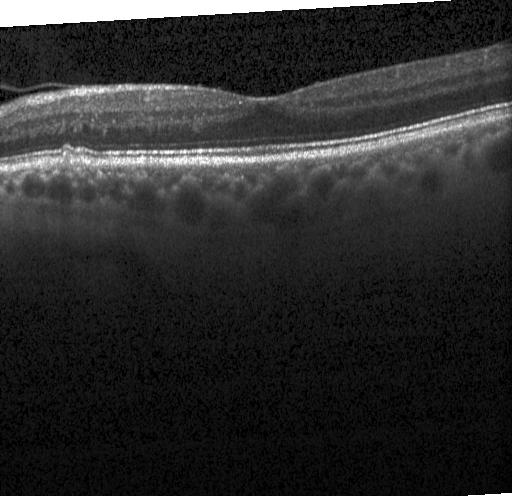 Horizontal scan through the fovea. Spectral-domain OCT. Retinal OCT B-scan. Sub-RPE drusenoid deposits.